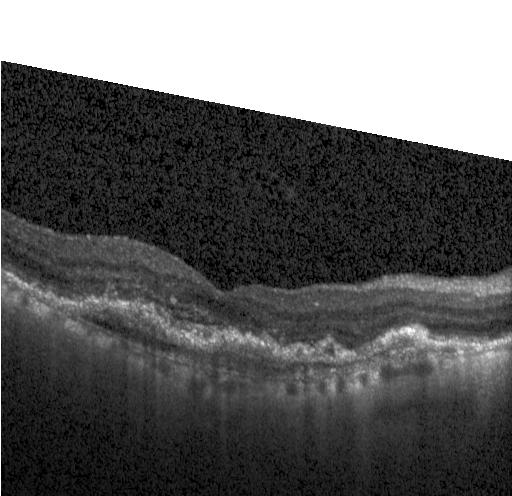
Macular OCT: a choroidal neovascular membrane.